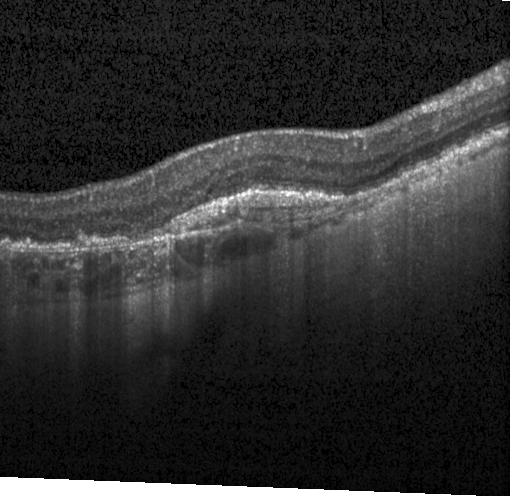
Impression: a choroidal neovascular membrane.